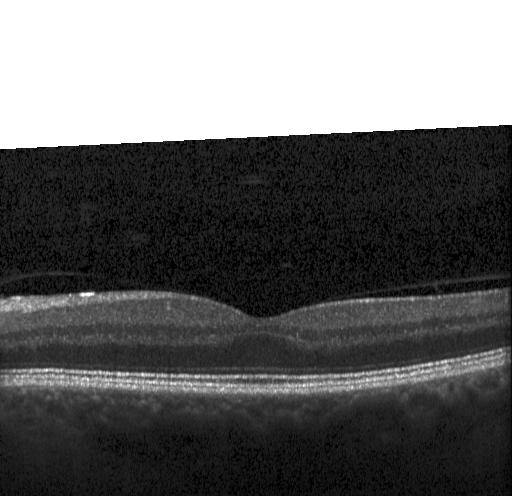
This B-scan demonstrates no choroidal neovascularization, diabetic macular edema, or drusen.